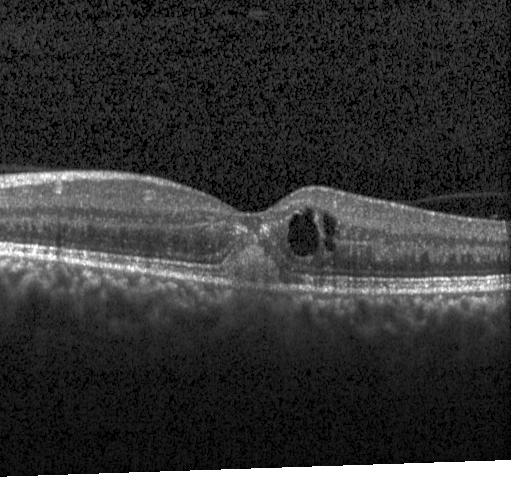 Heidelberg Spectralis. Retinal OCT cross-section. OCT finding: a choroidal neovascular membrane.